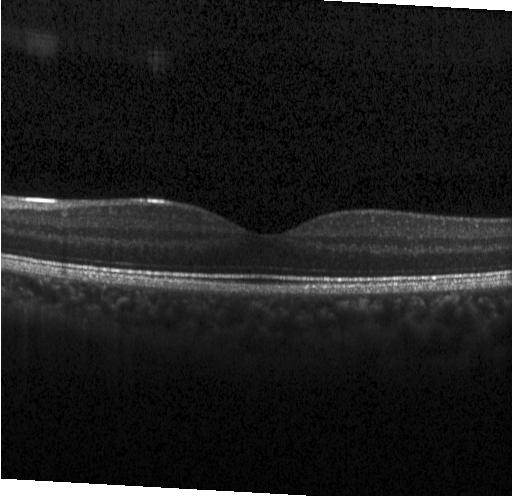 Diagnosis: no choroidal neovascularization, no diabetic macular edema, and no drusen.